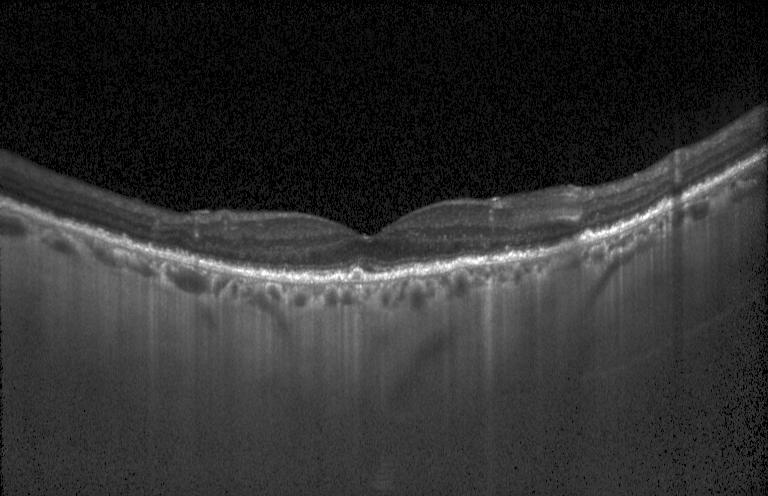

SD-OCT, through the macula, OCT B-scan
Diagnosis: drusen.